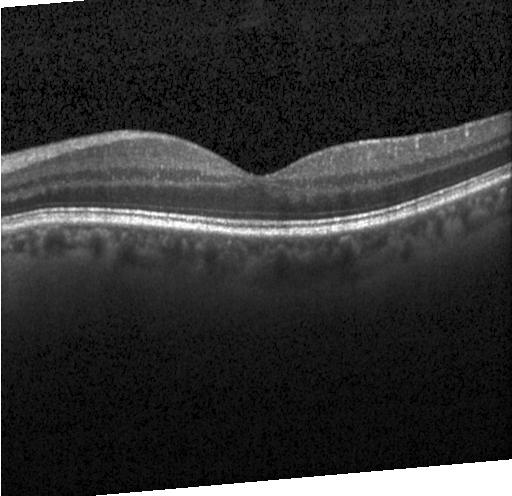
Impression: no CNV, no DME, and no drusen.